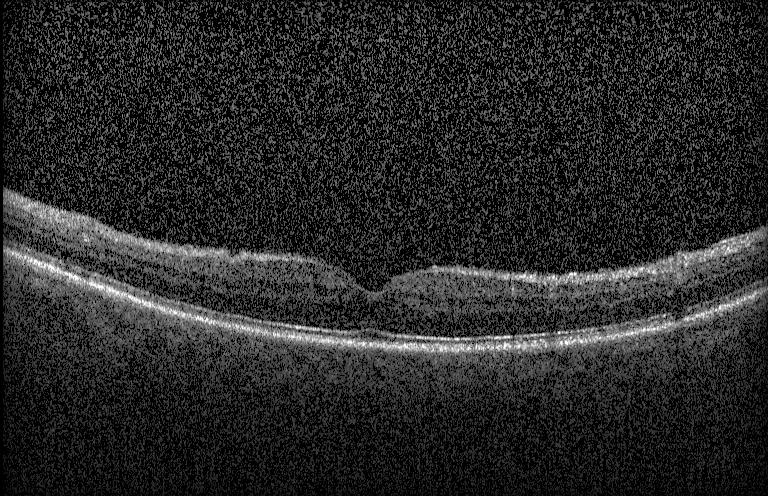
Heidelberg Spectralis. Spectral-domain optical coherence tomography. OCT line scan
Assessment: neither choroidal neovascularization, diabetic macular edema, nor drusen.